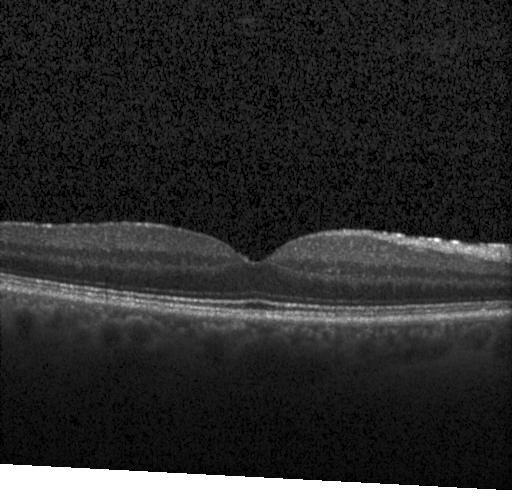

Spectral-domain optical coherence tomography · OCT B-scan · instrument: Heidelberg Spectralis · macular scan.
Finding: no CNV, DME, or drusen.